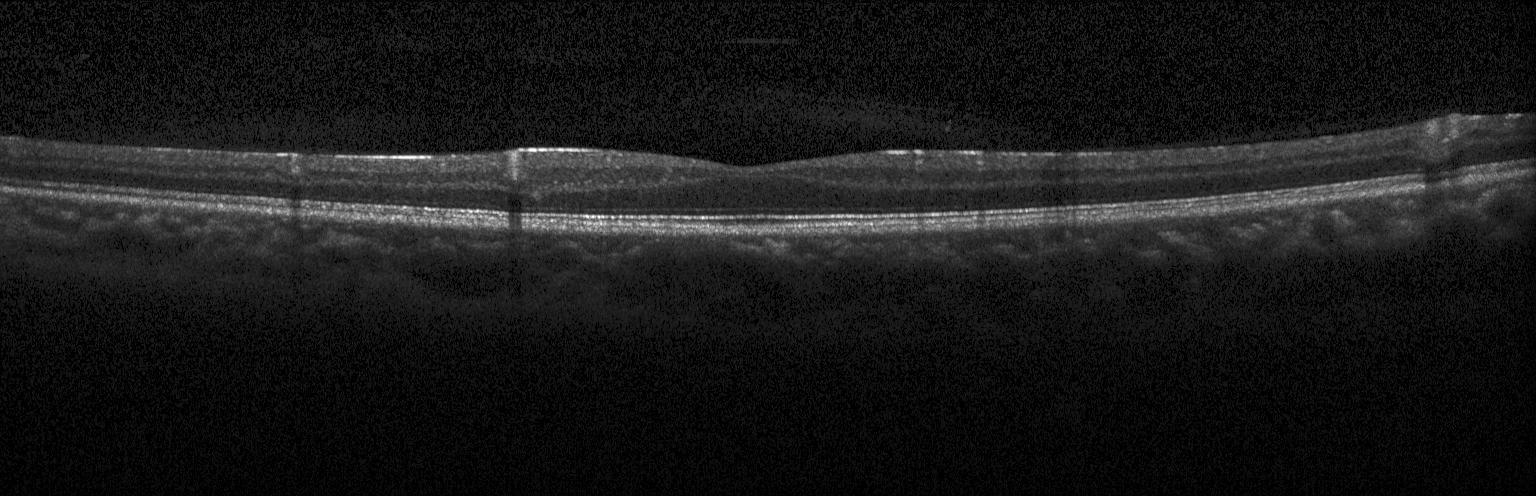

SD-OCT. Optical coherence tomography B-scan. Fovea-centered. Impression: no choroidal neovascularization, no diabetic macular edema, and no drusen.